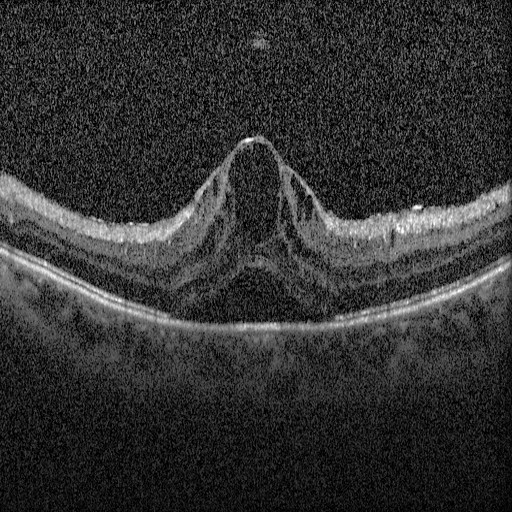
Horizontal scan through the fovea · retinal OCT cross-section — Finding: DME.